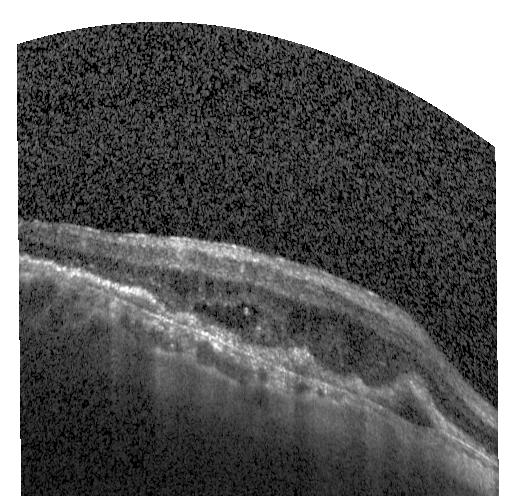
OCT B-scan showing a choroidal neovascular membrane.